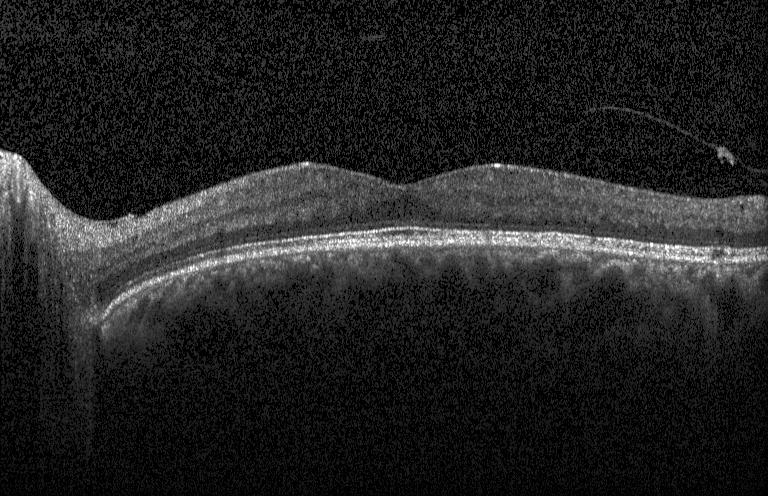 Diagnosis: no evidence of choroidal neovascularization, diabetic macular edema, or drusen.